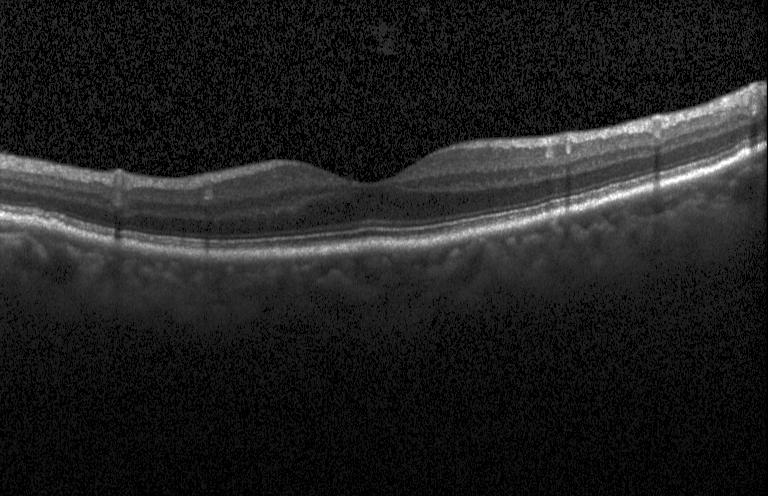

Instrument: Heidelberg Spectralis · horizontal scan through the fovea · optical coherence tomography scan · spectral-domain optical coherence tomography.
Dx: neither CNV, DME, nor drusen.